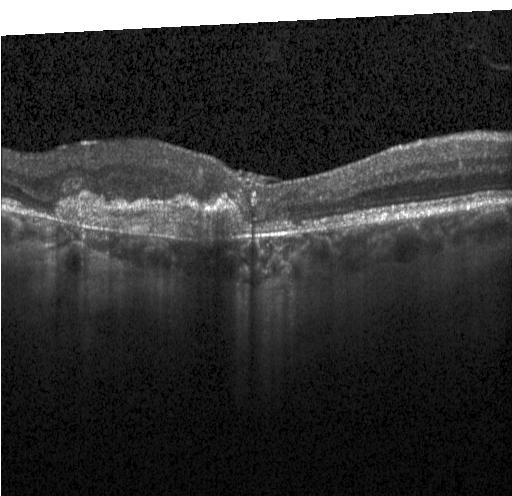 The scan shows a choroidal neovascular membrane.